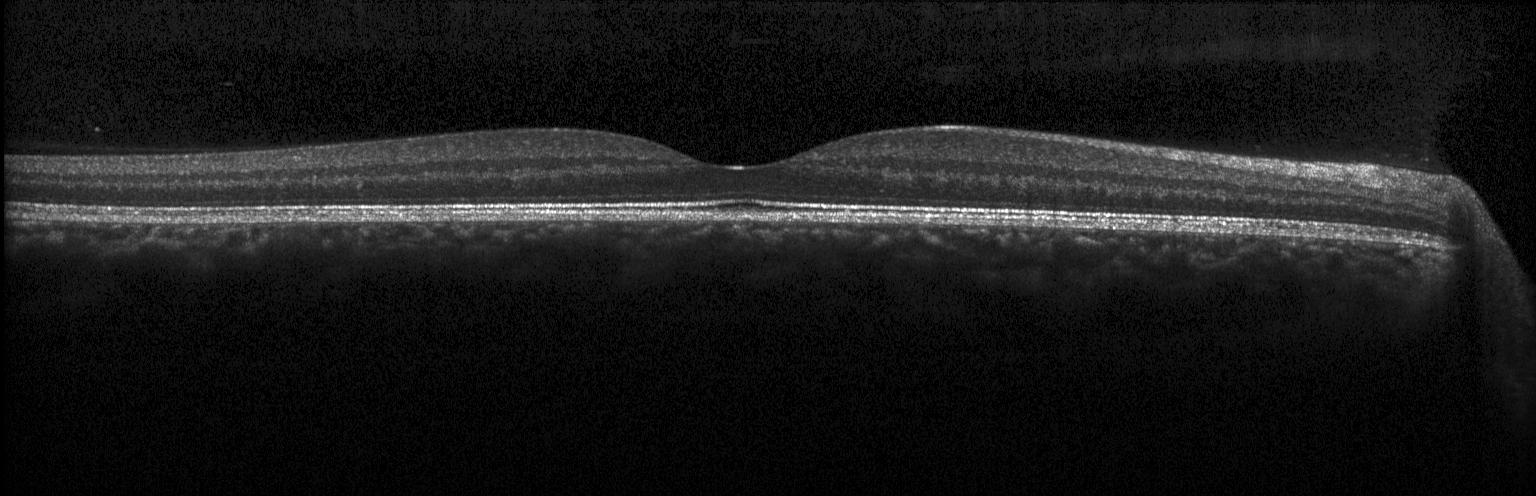 Horizontal scan through the fovea. Spectral-domain optical coherence tomography. Heidelberg Spectralis OCT system. OCT line scan. Assessment: no choroidal neovascularization, no diabetic macular edema, and no drusen.